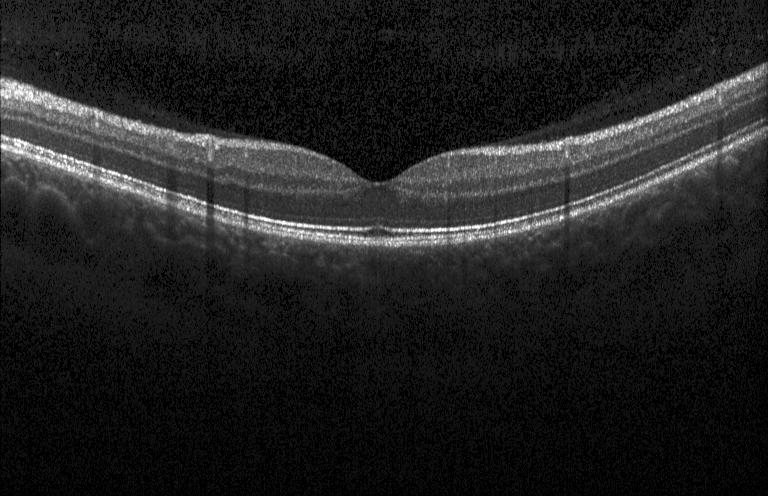 OCT B-scan · acquired on a Heidelberg Spectralis · spectral-domain optical coherence tomography.
Assessment: no choroidal neovascularization, no diabetic macular edema, and no drusen.